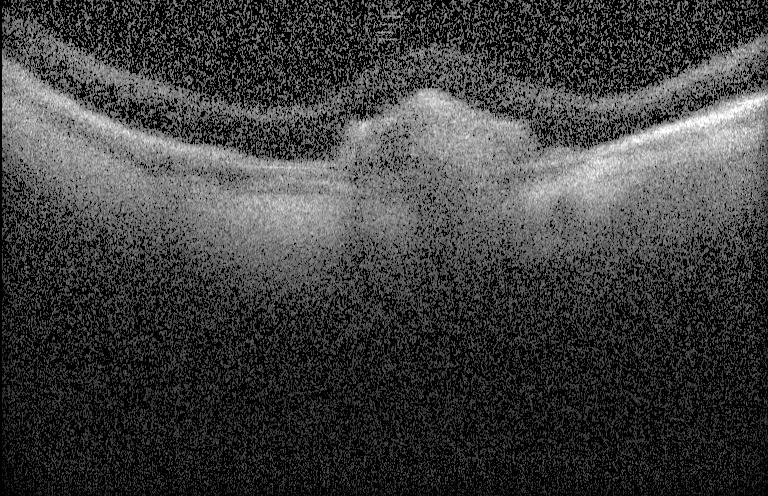

Retinal OCT cross-section — Finding: choroidal neovascularization.